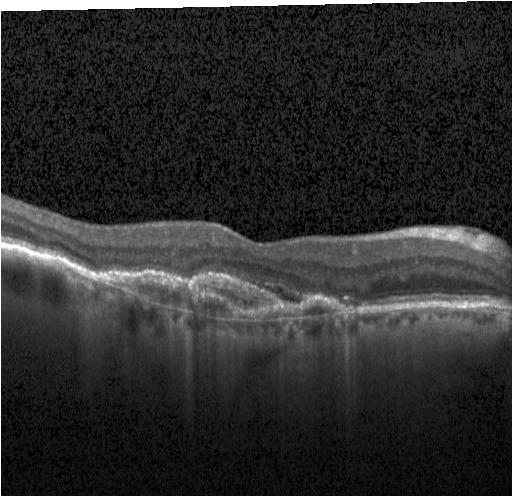 Macular OCT: a choroidal neovascular membrane.